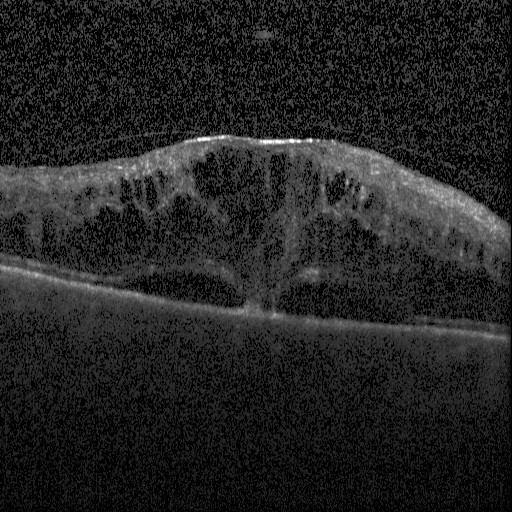

Retinal OCT cross-section. Impression: diabetic macular edema (DME).